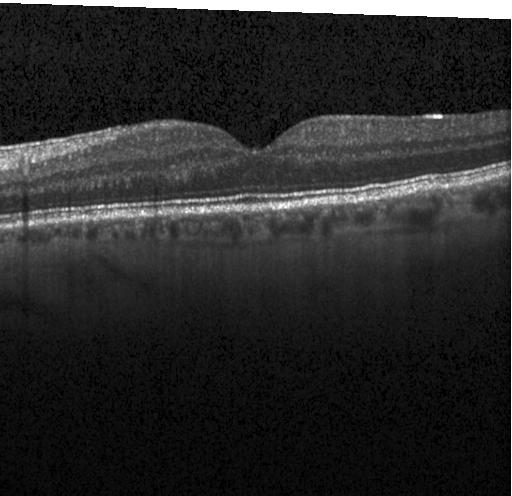
Acquired on a Heidelberg Spectralis; OCT line scan
Finding: no evidence of choroidal neovascularization, diabetic macular edema, or drusen.